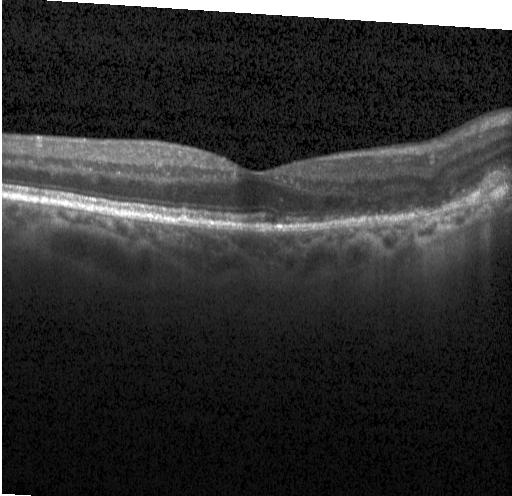

OCT finding: a choroidal neovascular membrane.